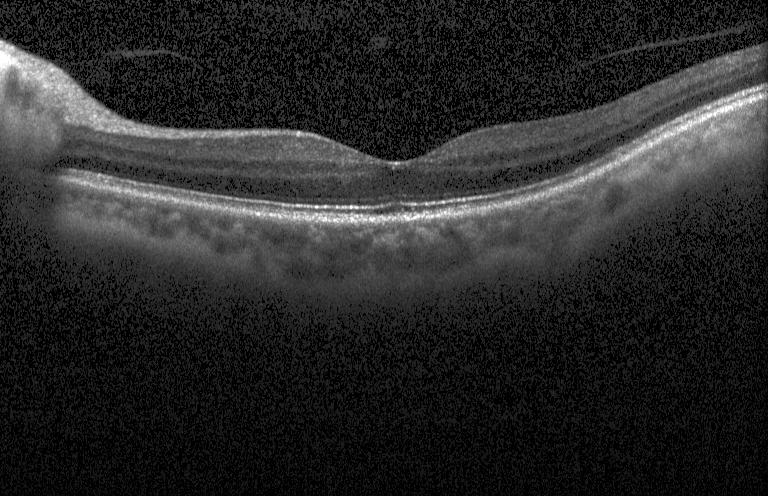
Spectral-domain optical coherence tomography; retinal OCT cross-section; fovea-centered; instrument: Heidelberg Spectralis — Macular OCT: no evidence of choroidal neovascularization, diabetic macular edema, or drusen.